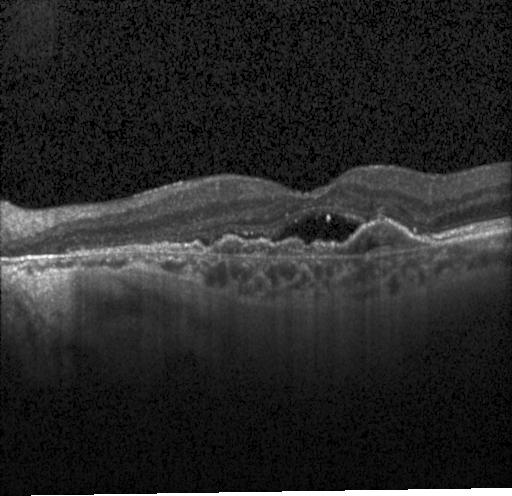

Macular OCT demonstrating choroidal neovascularization (CNV).